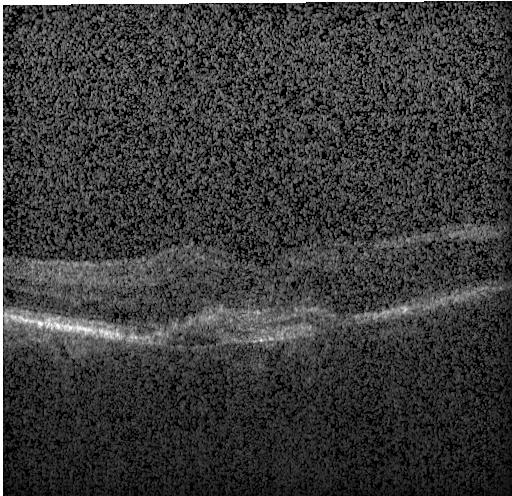 OCT B-scan, spectral-domain optical coherence tomography
Impression: a choroidal neovascular membrane.